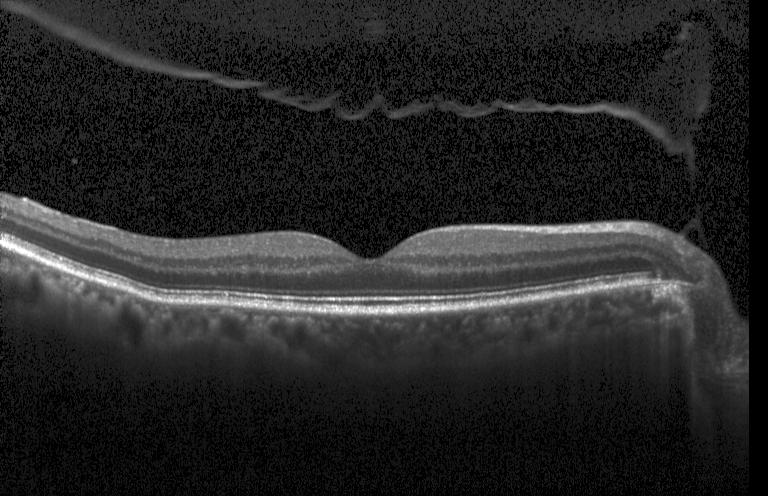
Macular scan; optical coherence tomography B-scan — Diagnosis: no evidence of CNV, DME, or drusen.